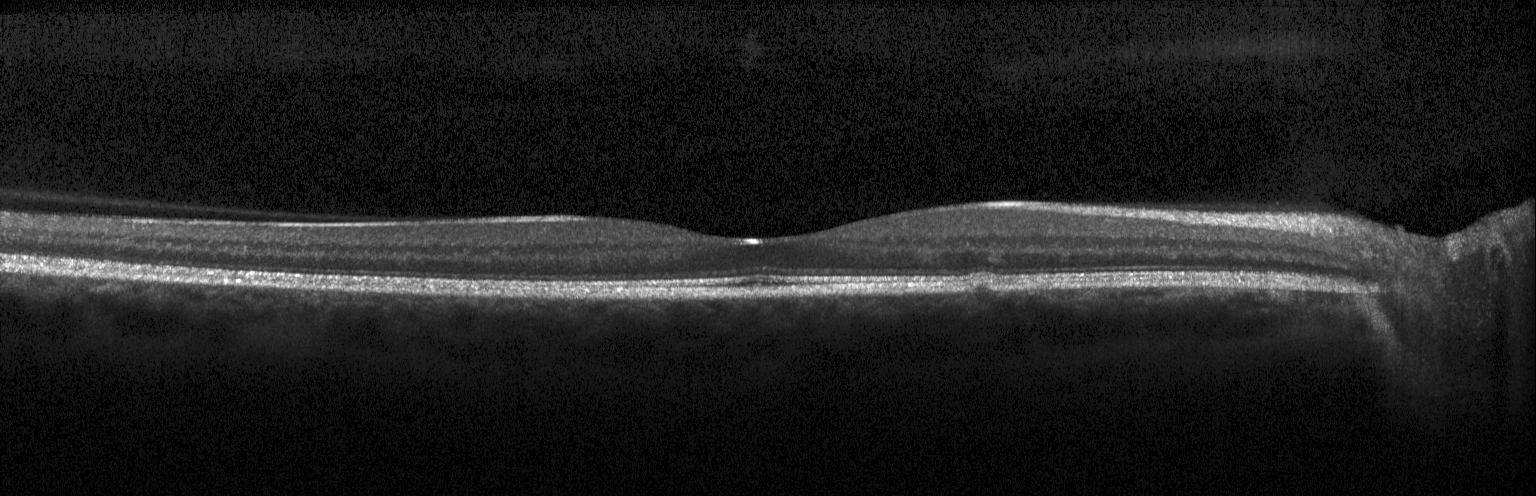 This B-scan demonstrates neither CNV, DME, nor drusen.